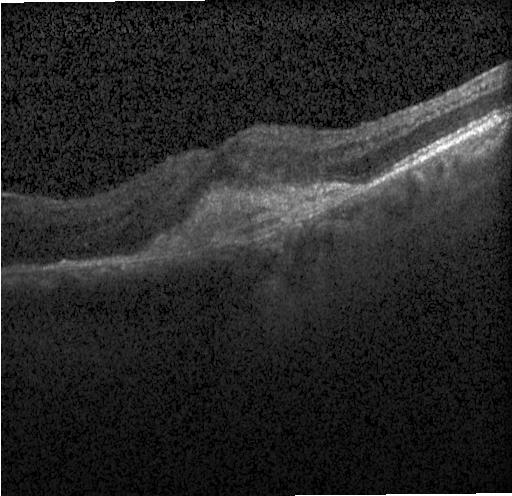
Spectral-domain optical coherence tomography; optical coherence tomography scan; centered on the fovea. Impression: a choroidal neovascular membrane.